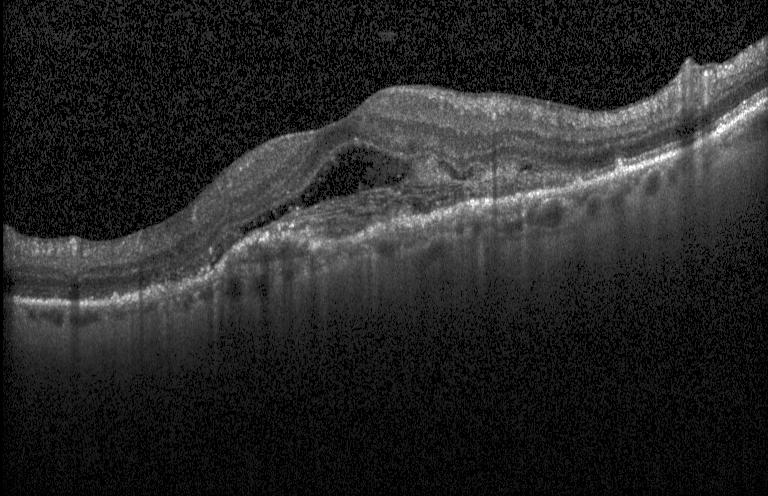 Retinal OCT cross-section showing a choroidal neovascular membrane.